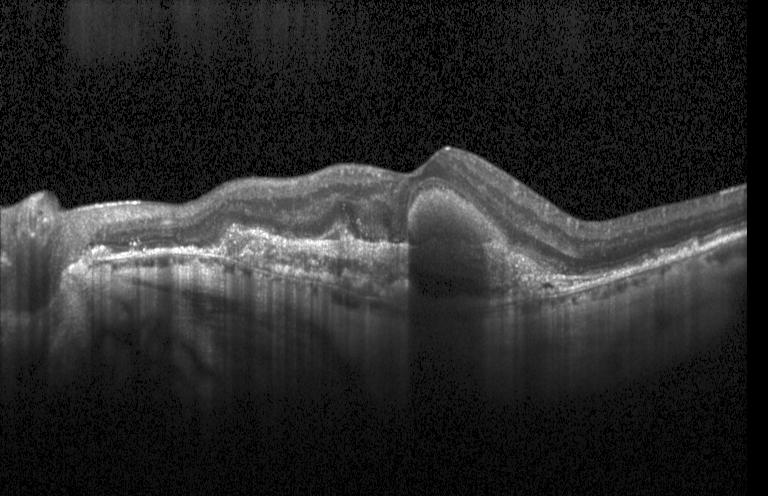

SD-OCT, optical coherence tomography scan, horizontal scan through the fovea, acquired on a Heidelberg Spectralis
Finding: a choroidal neovascular membrane.